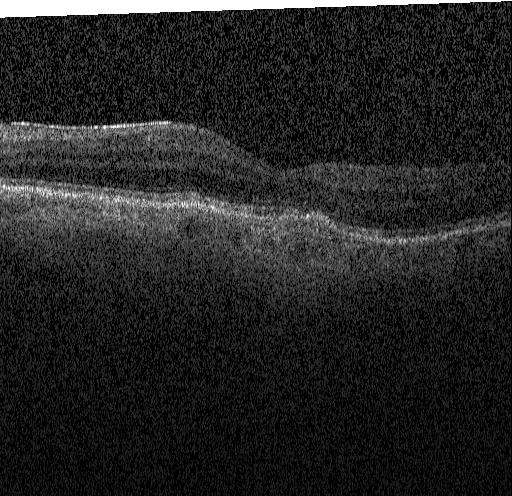
The scan shows CNV.